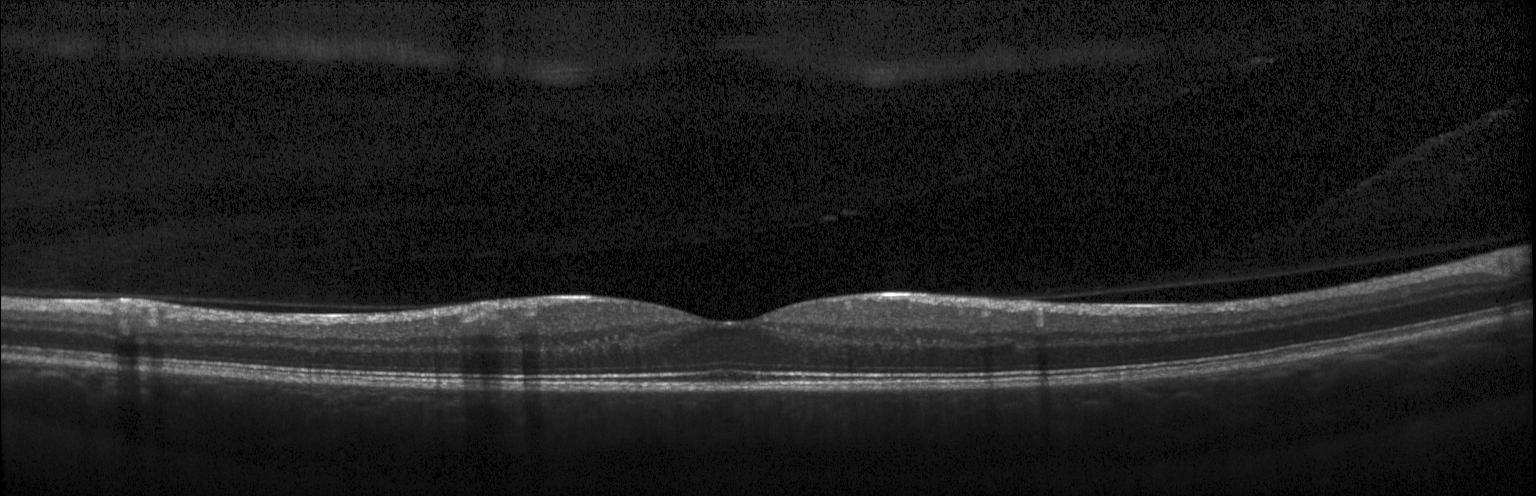

OCT line scan · centered on the fovea · acquired on a Heidelberg Spectralis. Diagnosis: no choroidal neovascularization, diabetic macular edema, or drusen.